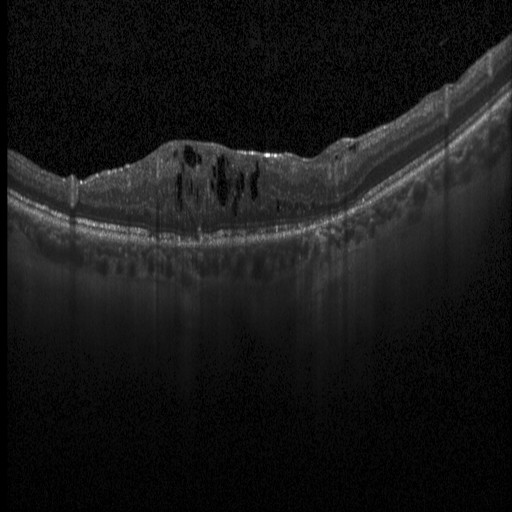

Spectral-domain OCT B-scan: diabetic macular edema.